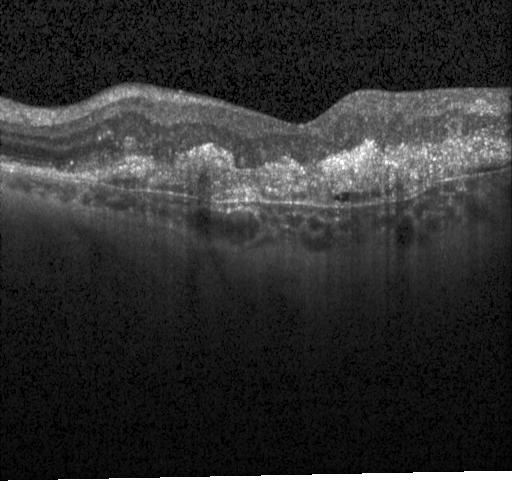
Retinal OCT B-scan, fovea-centered — The scan shows CNV.